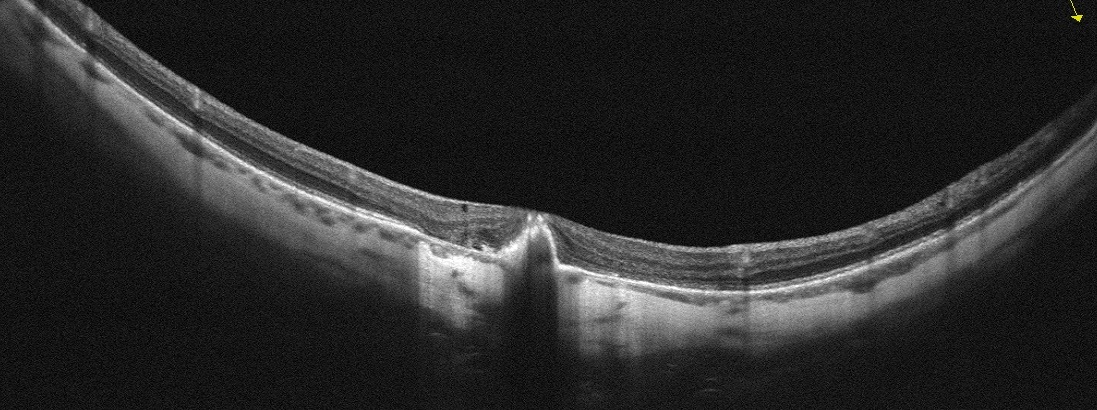 Optical coherence tomography B-scan
OCT finding: age-related macular degeneration (AMD).